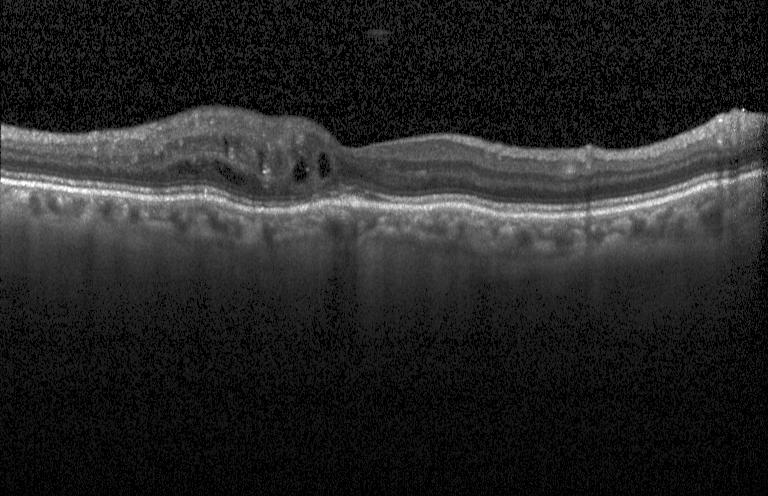 Impression: diabetic macular edema.